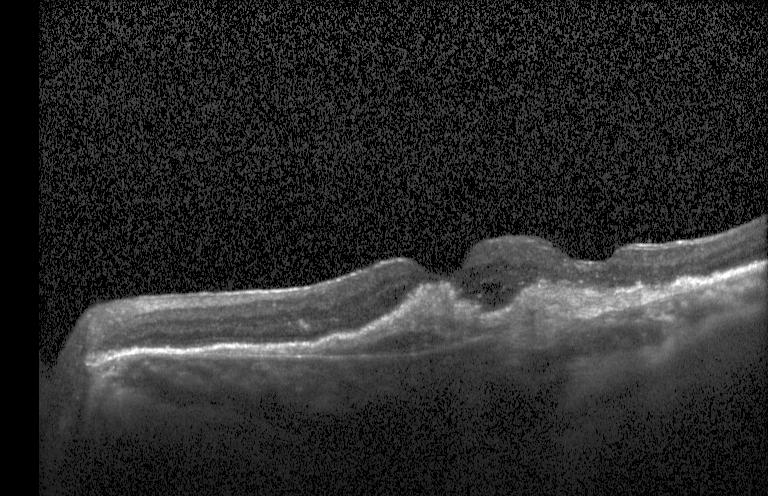

Spectral-domain OCT; acquired on a Heidelberg Spectralis; retinal OCT cross-section
OCT finding: choroidal neovascularization (CNV).